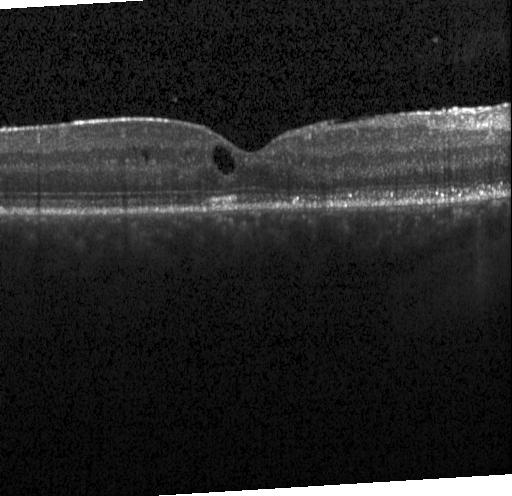

DME.